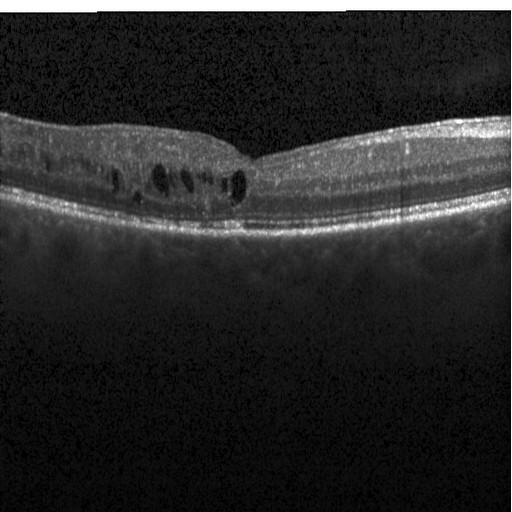 Heidelberg Spectralis · retinal OCT cross-section.
Impression: DME.